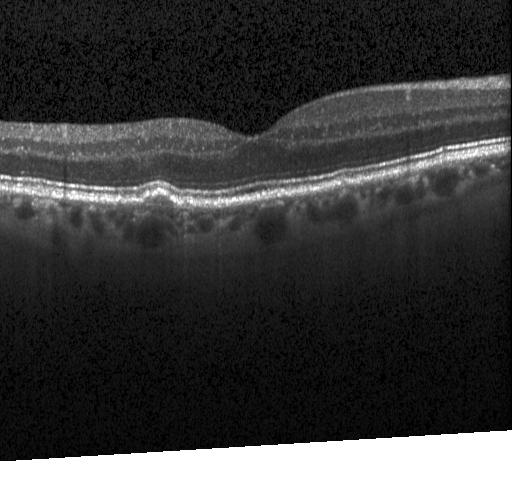 OCT line scan · instrument: Heidelberg Spectralis.
Impression: multiple drusen.